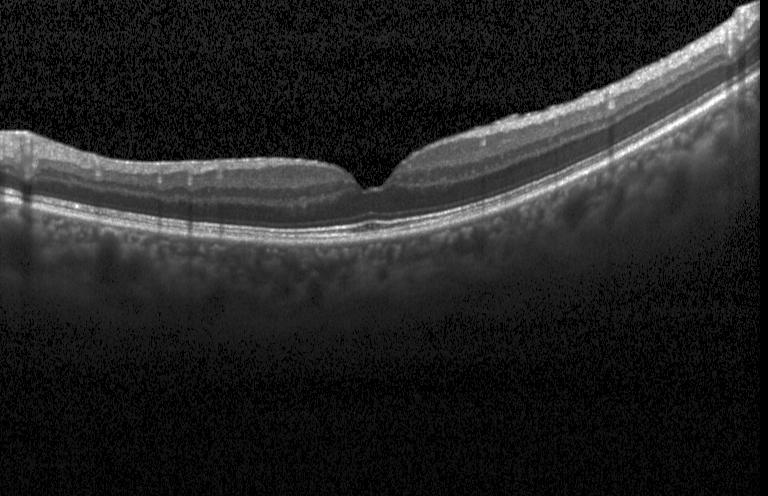

OCT B-scan — Assessment: no choroidal neovascularization, diabetic macular edema, or drusen.